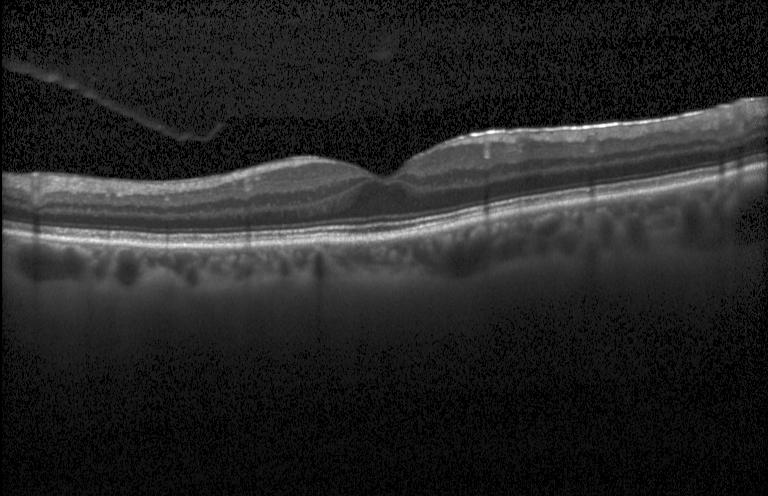 Impression: no evidence of choroidal neovascularization, diabetic macular edema, or drusen.